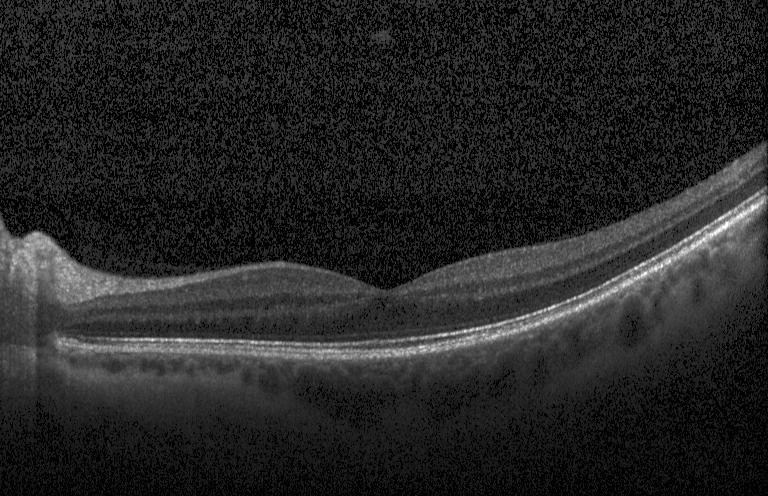

Spectral-domain optical coherence tomography; OCT line scan; horizontal scan through the fovea. Finding: no evidence of CNV, DME, or drusen.